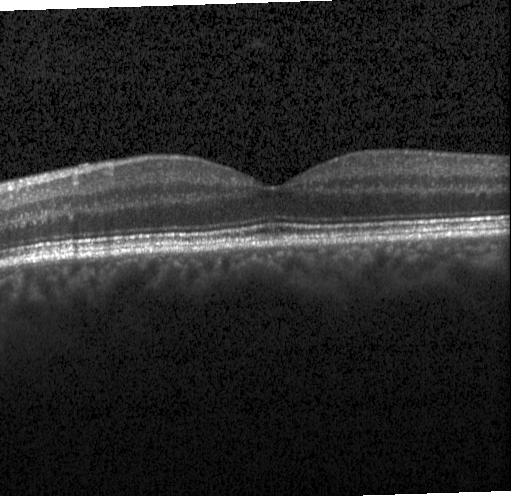
Acquired on a Heidelberg Spectralis · retinal OCT cross-section — The scan shows no choroidal neovascularization, no diabetic macular edema, and no drusen.